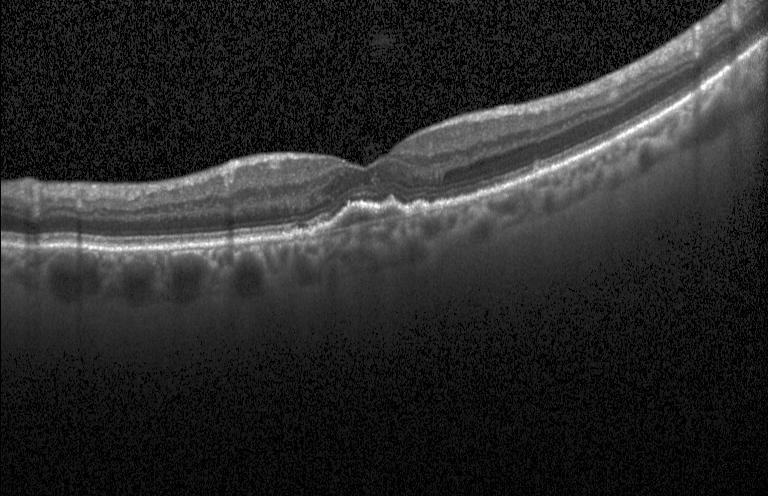

Retinal OCT cross-section, acquired on a Heidelberg Spectralis, SD-OCT, through the macula
CNV.